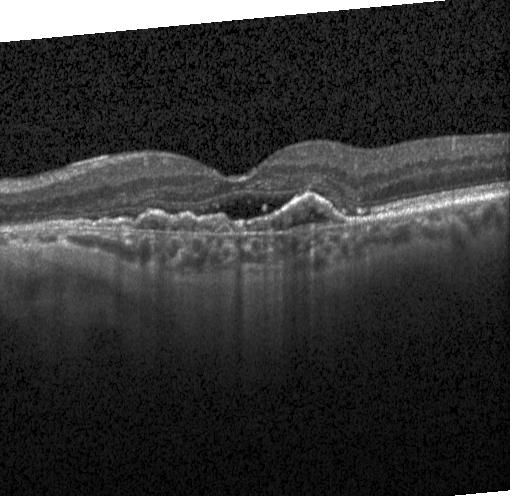
Optical coherence tomography B-scan. Instrument: Heidelberg Spectralis. Through the macula.
Dx: choroidal neovascularization.